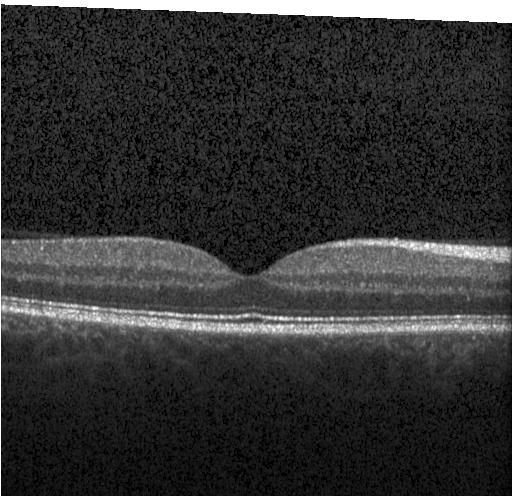

Assessment: no choroidal neovascularization, diabetic macular edema, or drusen.